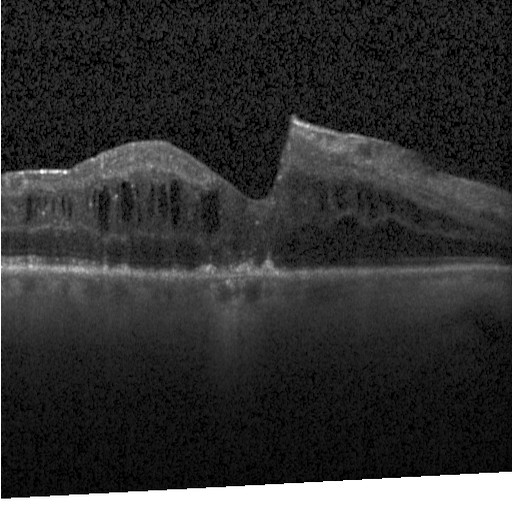
OCT line scan; spectral-domain OCT; horizontal scan through the fovea; Heidelberg Spectralis
Finding: diabetic macular edema.